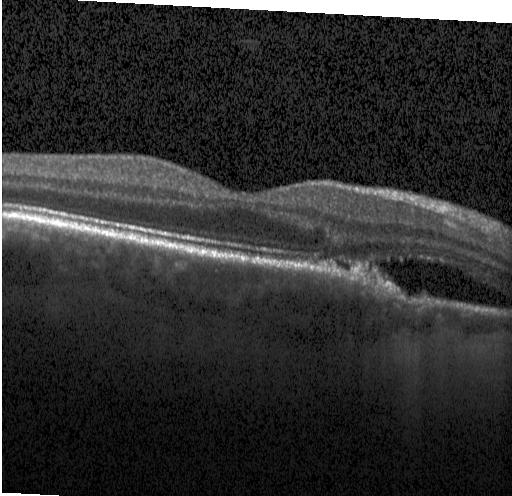 Diagnosis: a choroidal neovascular membrane.